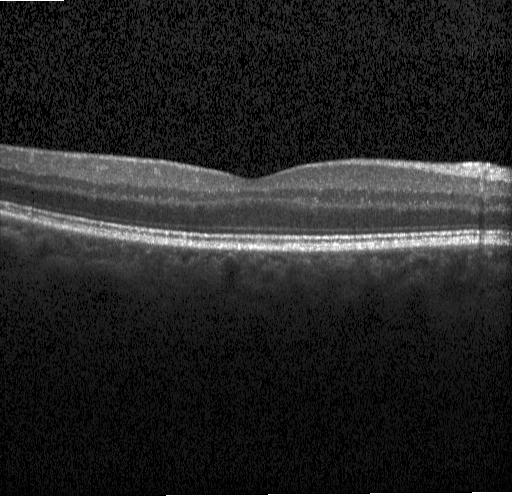
Retinal OCT cross-section, fovea-centered, spectral-domain OCT. Assessment: no choroidal neovascularization, diabetic macular edema, or drusen.